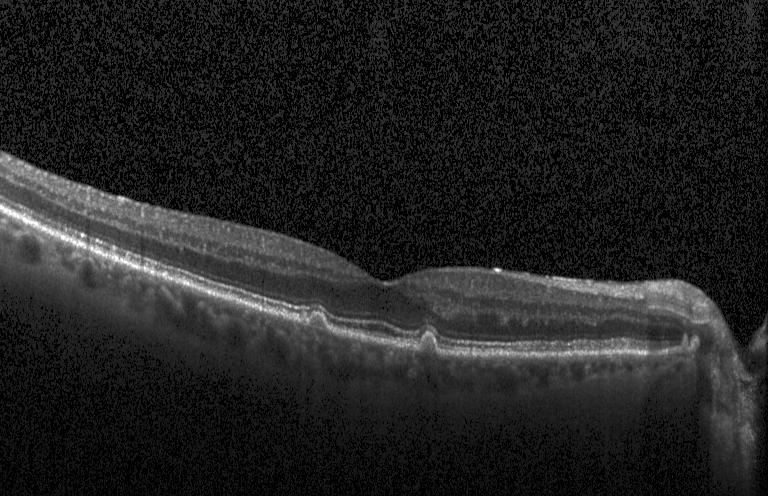

OCT B-scan
Dx: sub-RPE drusenoid deposits.